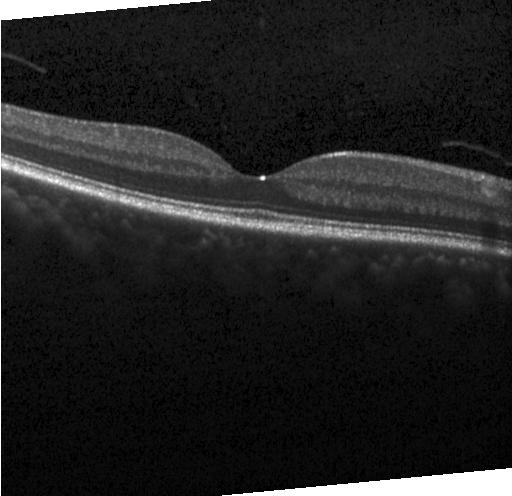 No choroidal neovascularization, no diabetic macular edema, and no drusen.